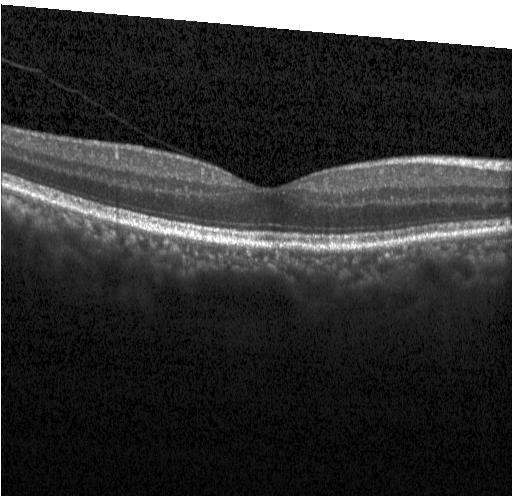 The scan shows no choroidal neovascularization, diabetic macular edema, or drusen.